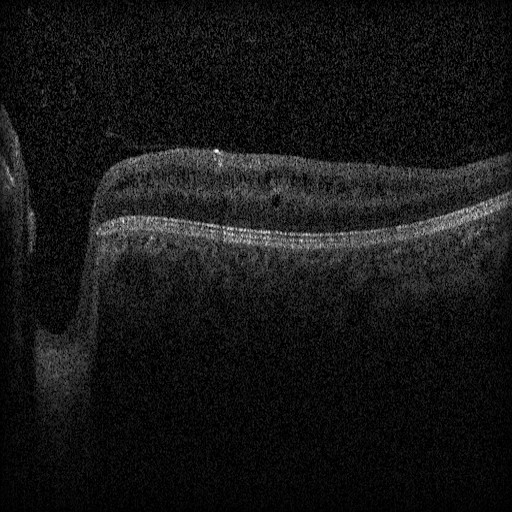 SD-OCT. OCT B-scan. Through the macula.
Macular OCT: DME.